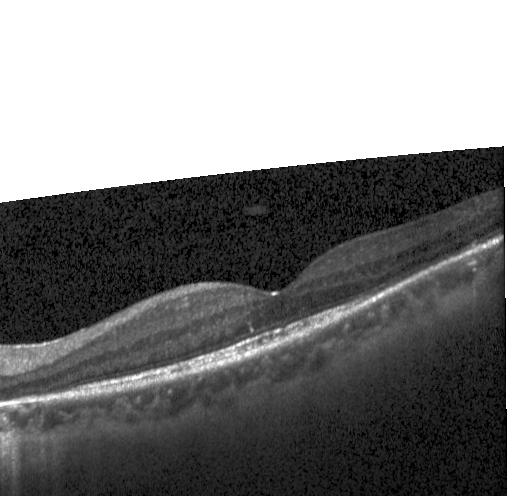
Retinal OCT cross-section. Centered on the fovea. Heidelberg Spectralis OCT system. Macular OCT: no evidence of choroidal neovascularization, diabetic macular edema, or drusen.